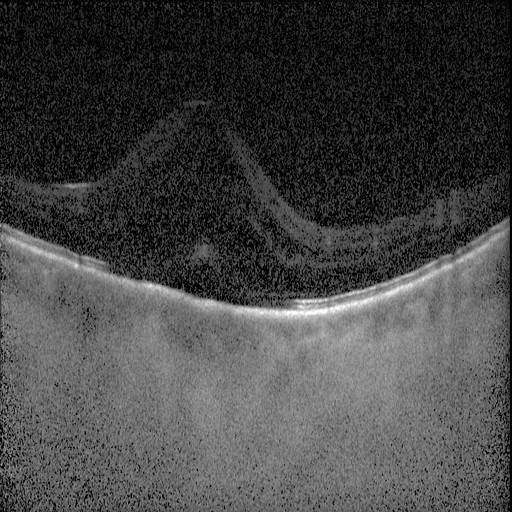
Centered on the fovea, retinal OCT cross-section.
Finding: diabetic macular edema.